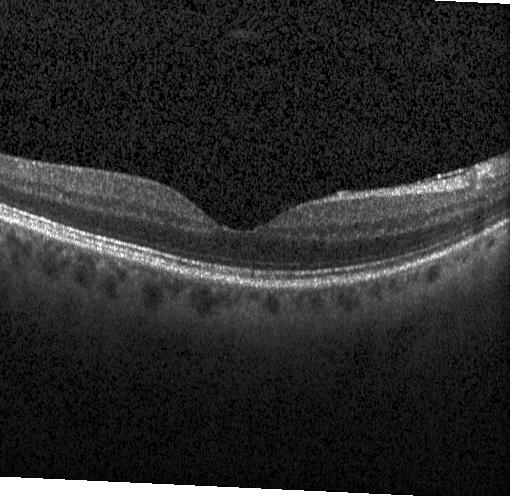
This B-scan demonstrates no choroidal neovascularization, diabetic macular edema, or drusen.